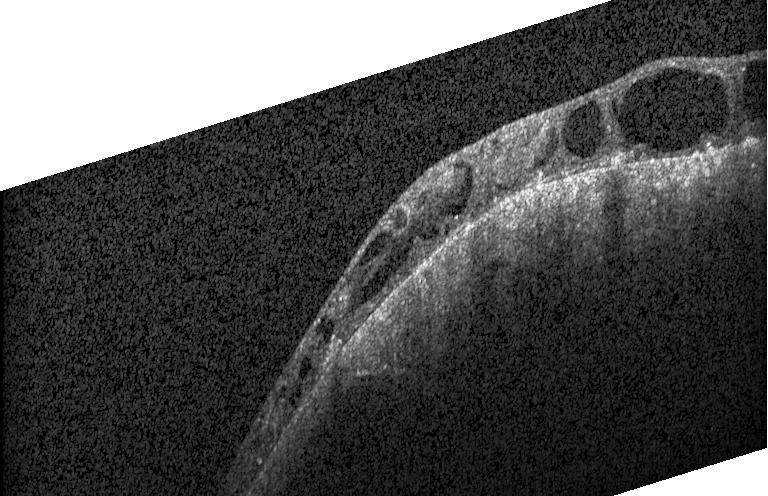
Optical coherence tomography scan. Diabetic macular edema.